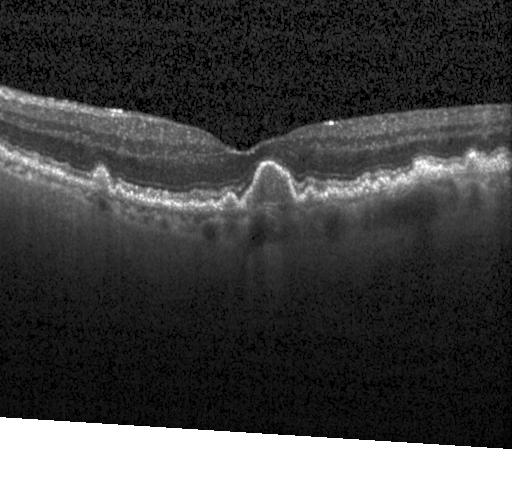

The scan shows multiple drusen.